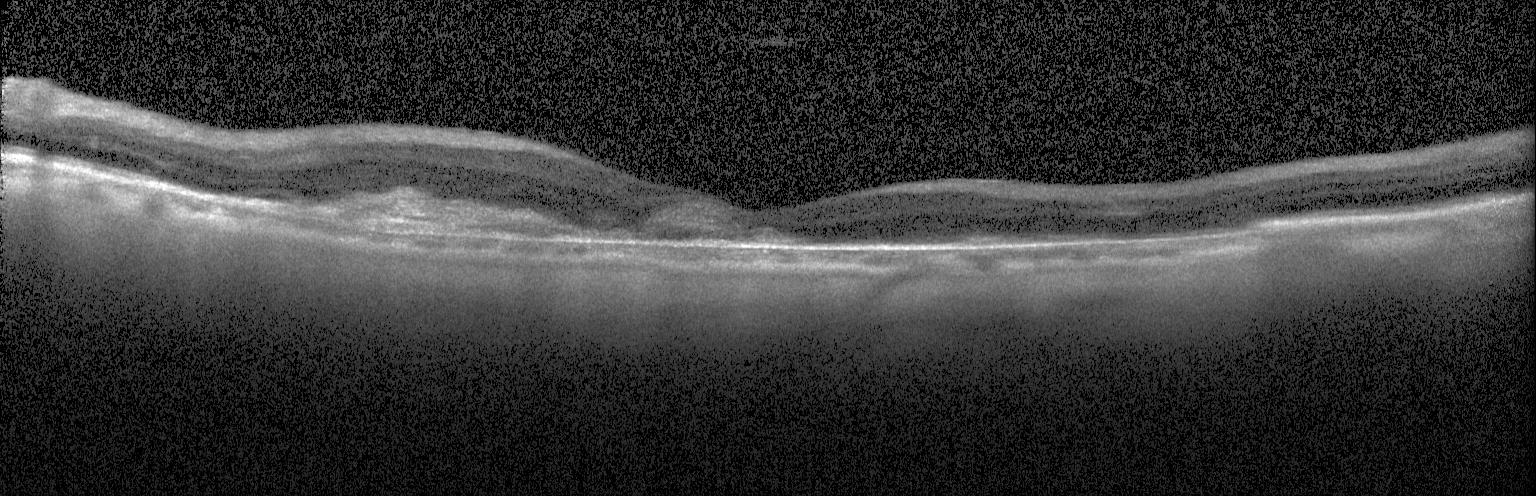

Optical coherence tomography B-scan; acquired on a Heidelberg Spectralis
Assessment: choroidal neovascularization (CNV).